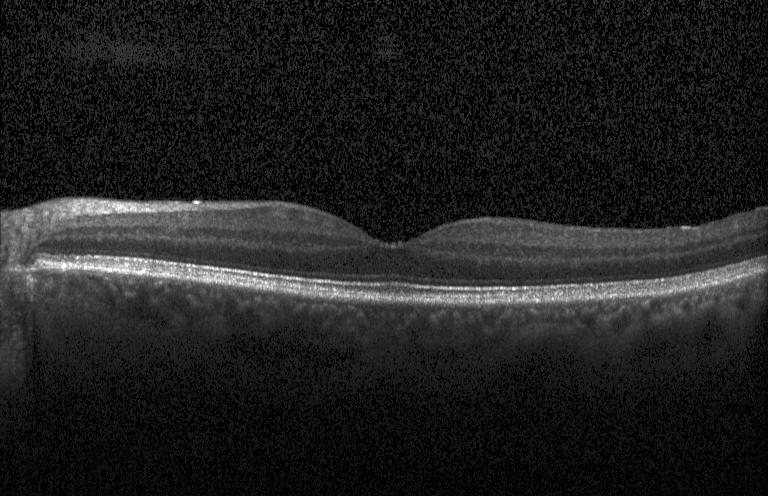

Retinal OCT B-scan — OCT finding: no choroidal neovascularization, no diabetic macular edema, and no drusen.